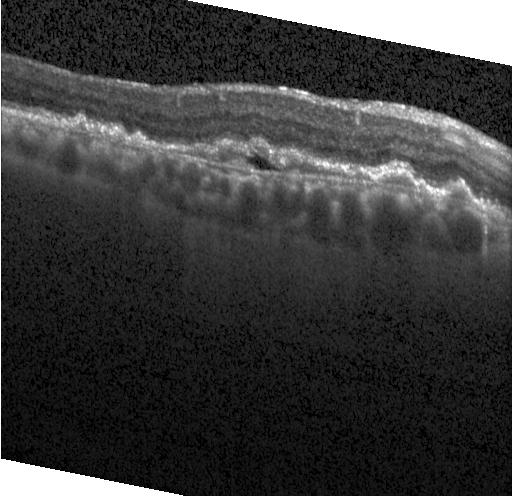

Spectral-domain OCT. OCT B-scan — Diagnosis: a choroidal neovascular membrane.